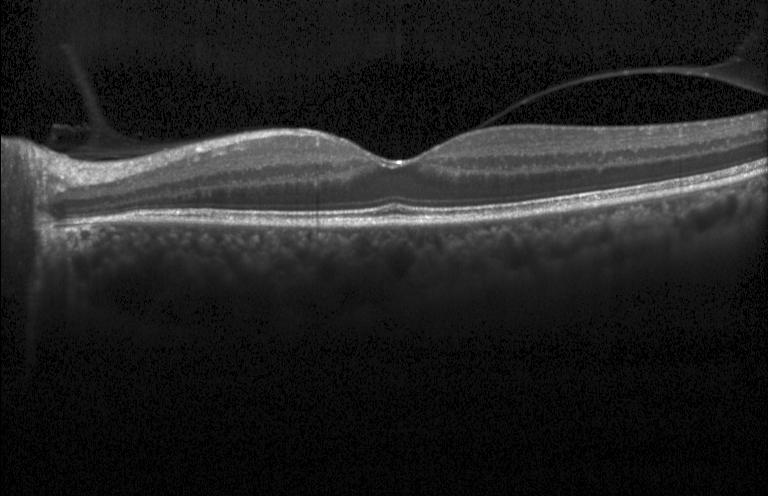
Retinal OCT B-scan; spectral-domain optical coherence tomography. Macular OCT: neither choroidal neovascularization, diabetic macular edema, nor drusen.